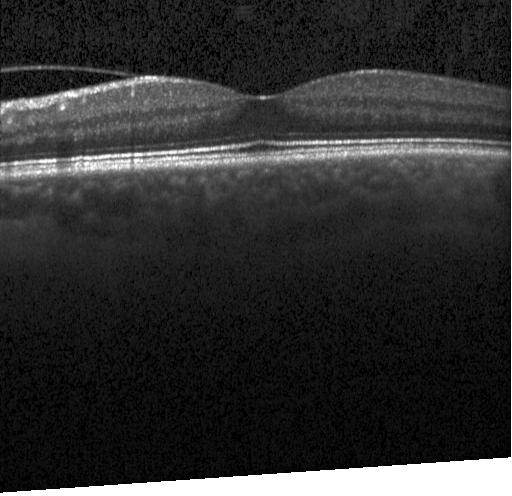 Spectral-domain OCT; OCT B-scan. OCT finding: no choroidal neovascularization, no diabetic macular edema, and no drusen.